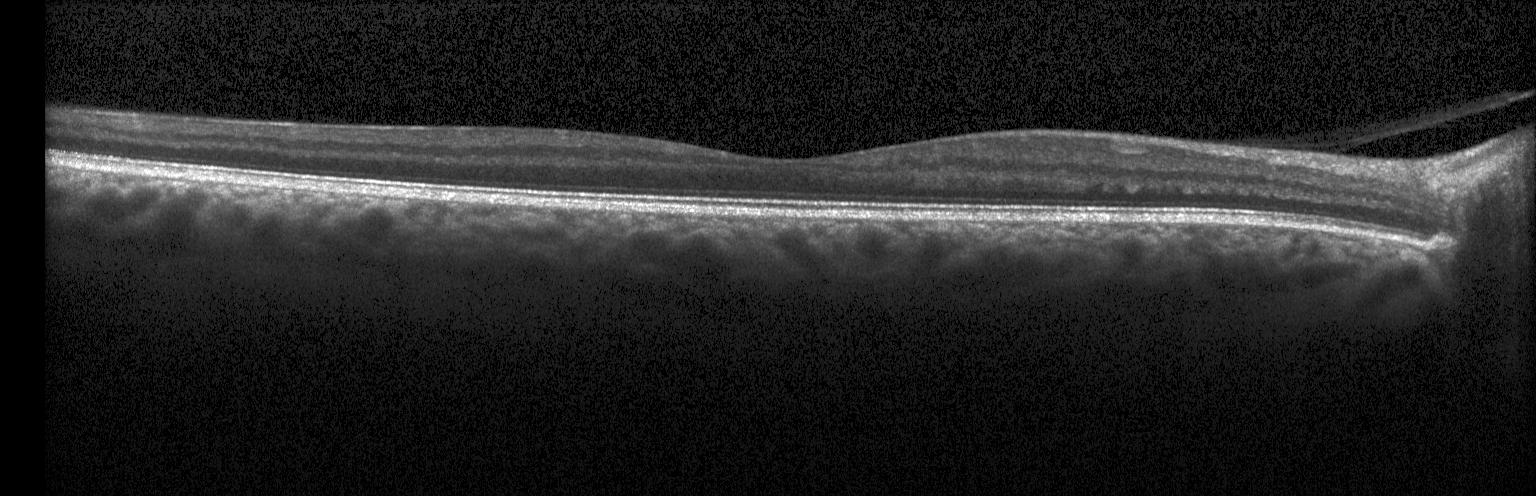 Diagnosis: no evidence of choroidal neovascularization, diabetic macular edema, or drusen.